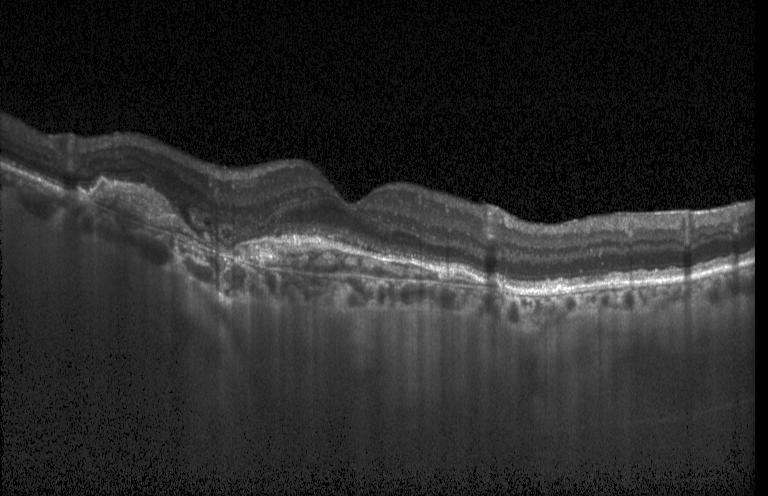
Dx: CNV.